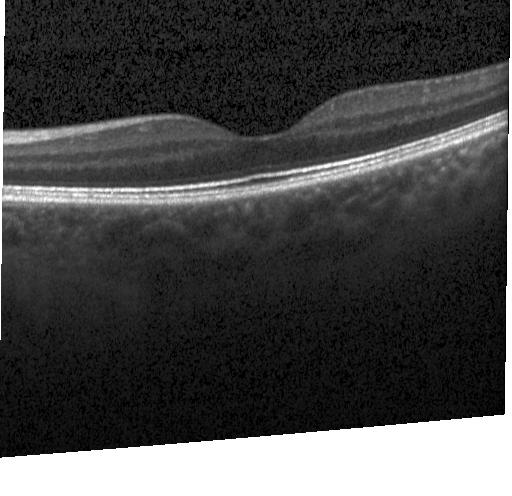

Optical coherence tomography B-scan. Instrument: Heidelberg Spectralis. Fovea-centered. Impression: no CNV, DME, or drusen.